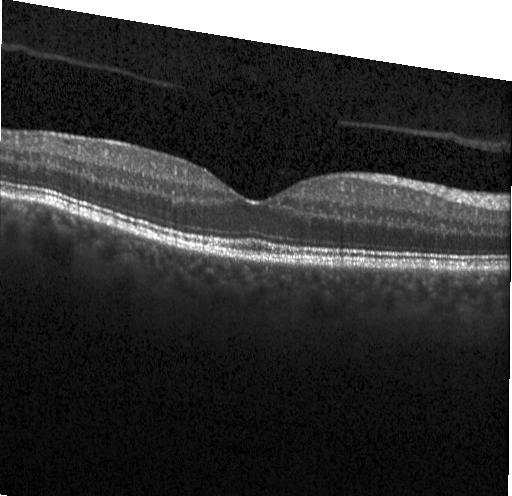
Optical coherence tomography B-scan; instrument: Heidelberg Spectralis — This B-scan demonstrates no evidence of choroidal neovascularization, diabetic macular edema, or drusen.